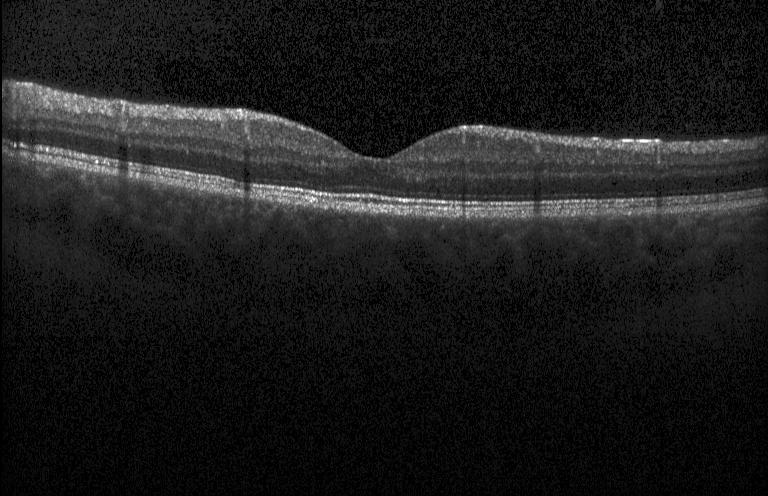 Macular OCT demonstrating neither CNV, DME, nor drusen.